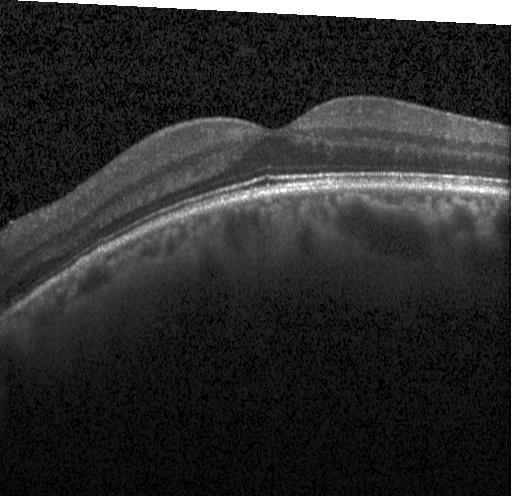

Optical coherence tomography scan · Heidelberg Spectralis · through the macula · SD-OCT
Assessment: no choroidal neovascularization, diabetic macular edema, or drusen.